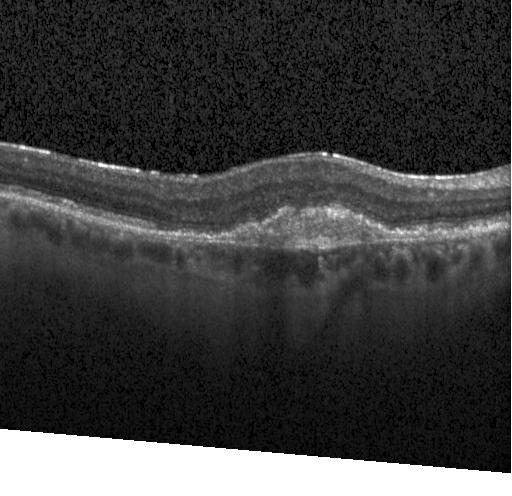
Centered on the fovea, optical coherence tomography scan, Heidelberg Spectralis OCT system
Impression: choroidal neovascularization (CNV).